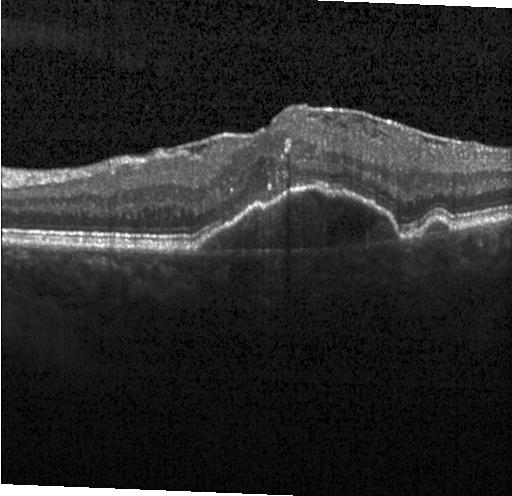
Heidelberg Spectralis · OCT line scan. OCT finding: CNV.